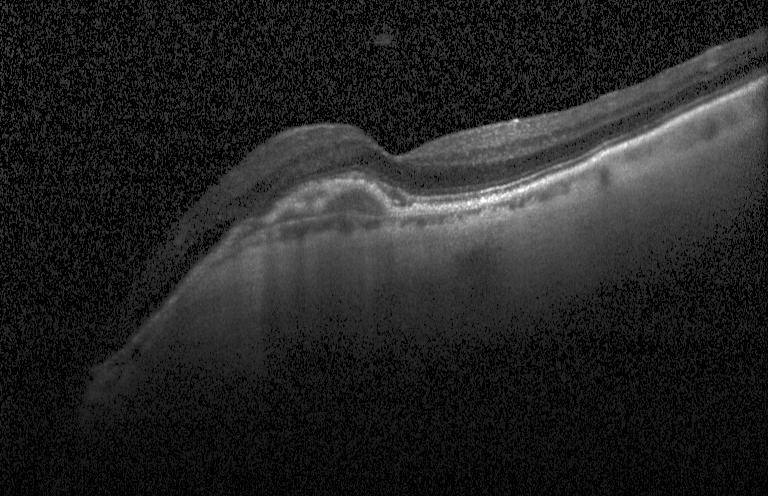

OCT scan showing choroidal neovascularization.